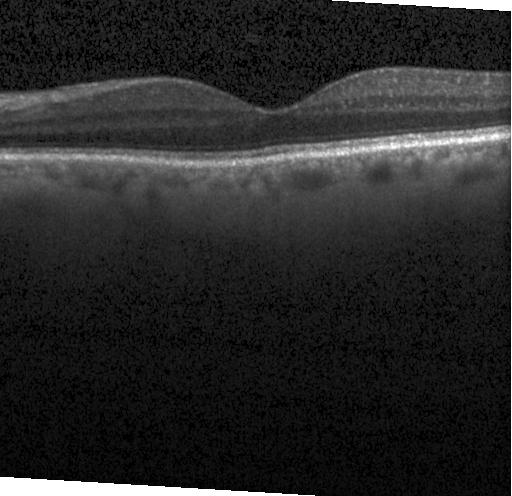
Retinal OCT B-scan. Diagnosis: no evidence of choroidal neovascularization, diabetic macular edema, or drusen.